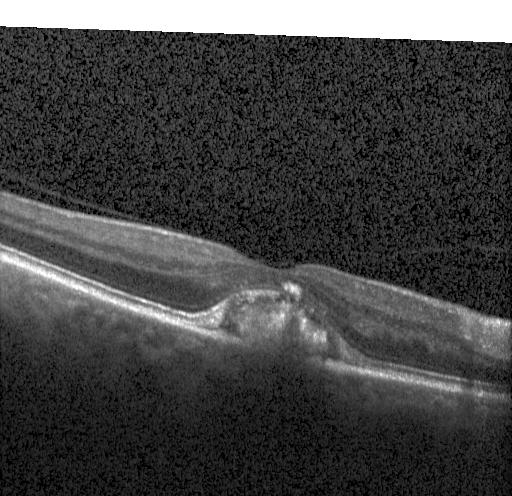
Centered on the fovea · acquired on a Heidelberg Spectralis · OCT B-scan
Macular OCT: a choroidal neovascular membrane.